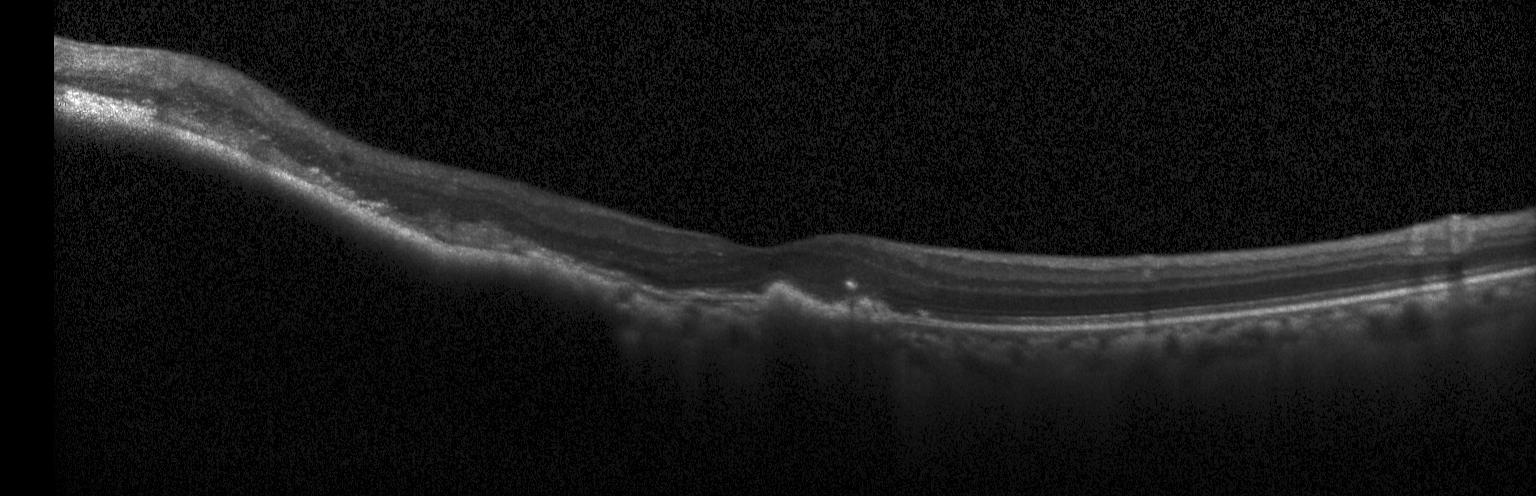 OCT B-scan. Finding: CNV.